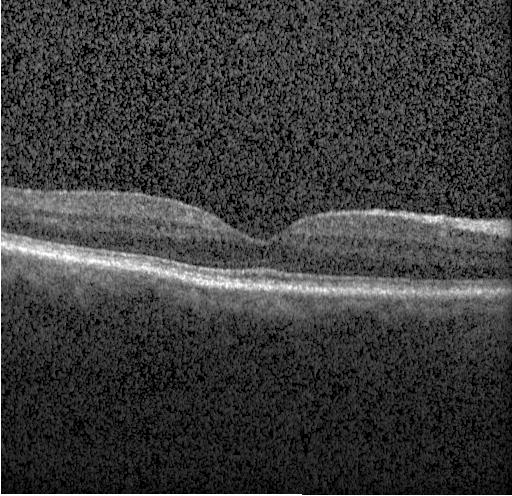

OCT B-scan; centered on the fovea; spectral-domain optical coherence tomography; acquired on a Heidelberg Spectralis. Diagnosis: no CNV, no DME, and no drusen.